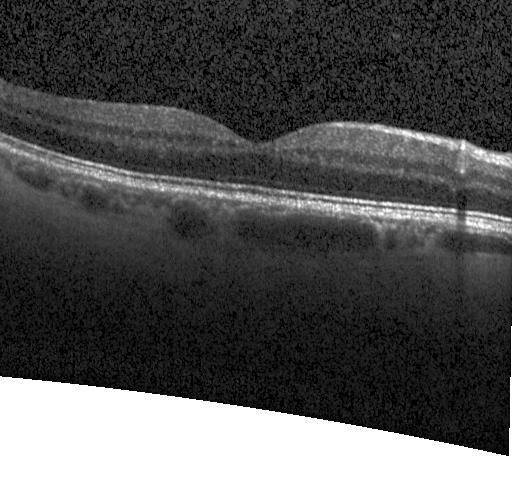 No choroidal neovascularization, no diabetic macular edema, and no drusen.